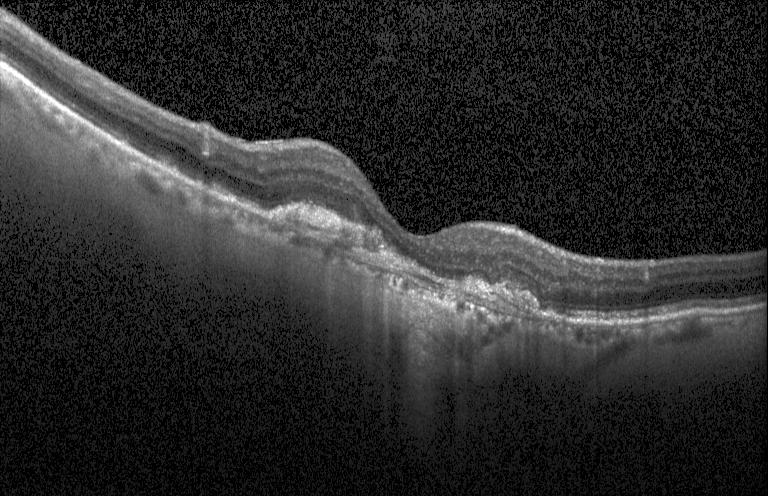
OCT line scan · macular scan
Impression: a choroidal neovascular membrane.